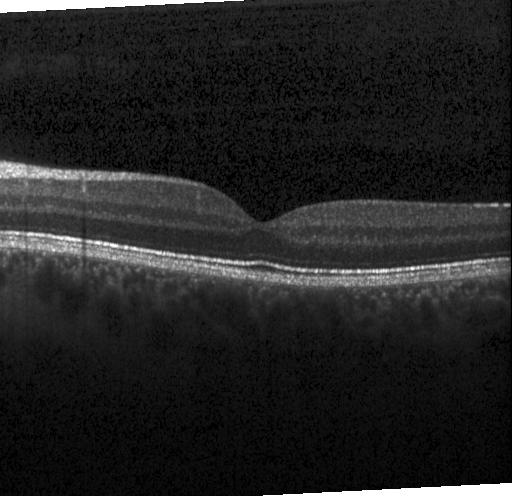

Heidelberg Spectralis OCT system; OCT B-scan — Finding: no choroidal neovascularization, diabetic macular edema, or drusen.